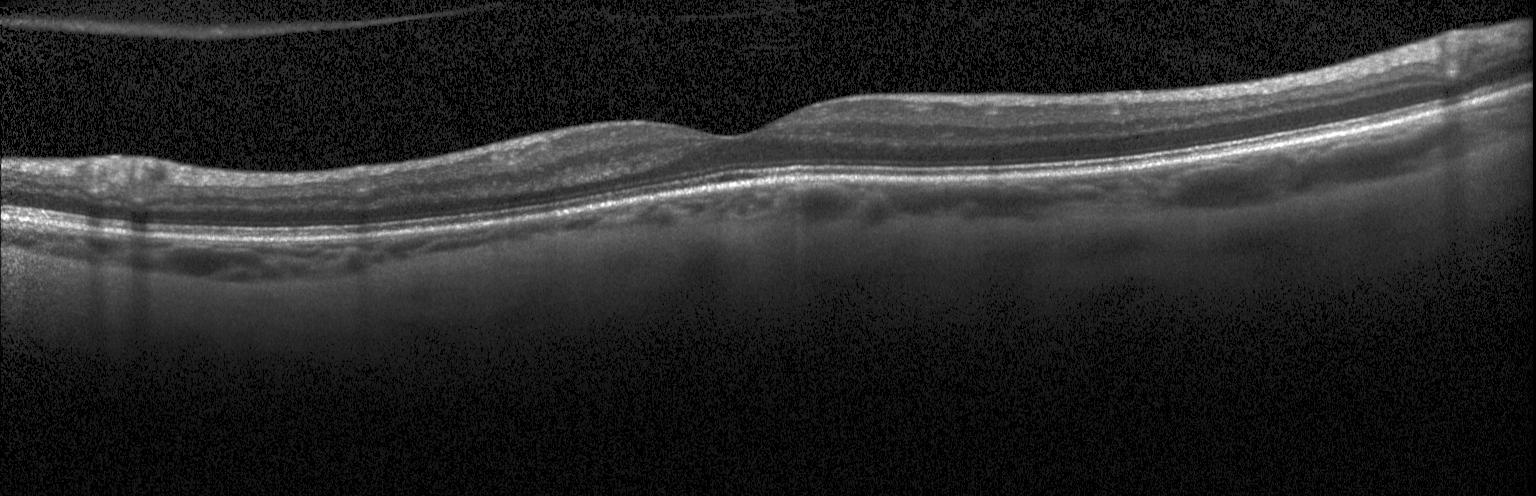 Diagnosis: no choroidal neovascularization, diabetic macular edema, or drusen.